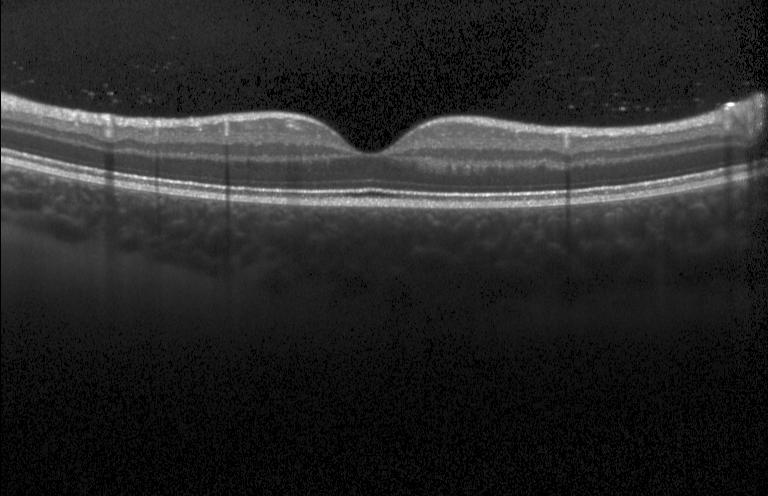

OCT line scan, spectral-domain optical coherence tomography
OCT finding: neither CNV, DME, nor drusen.